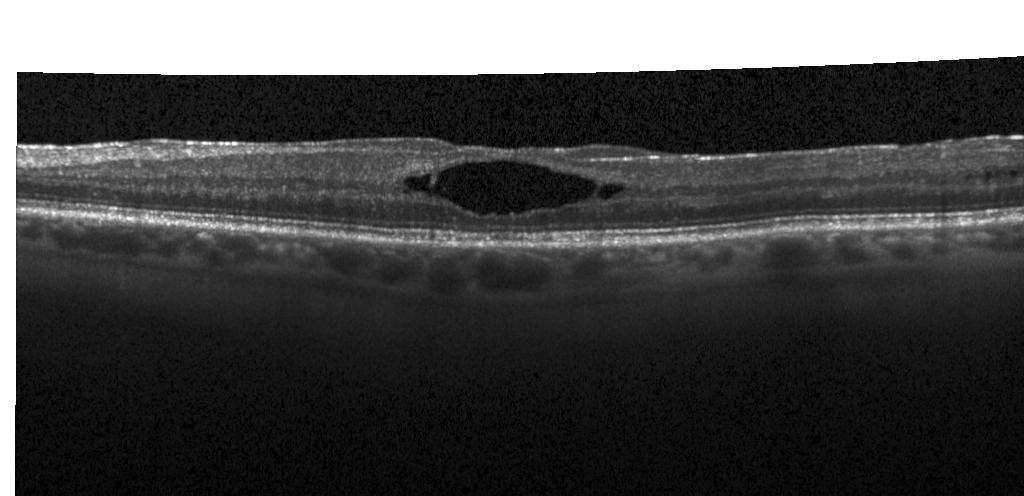
Retinal OCT B-scan, fovea-centered, Heidelberg Spectralis, spectral-domain OCT. Diabetic macular edema.